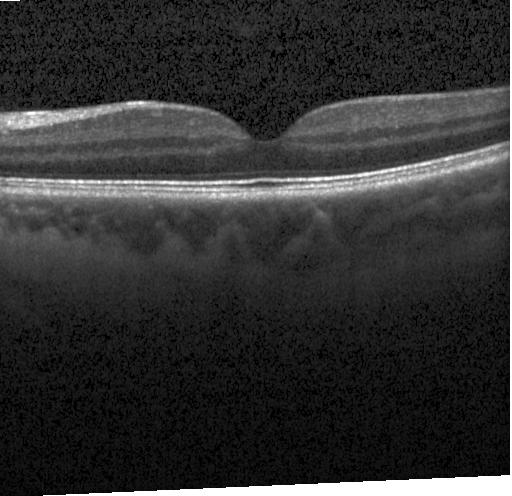
No choroidal neovascularization, diabetic macular edema, or drusen.